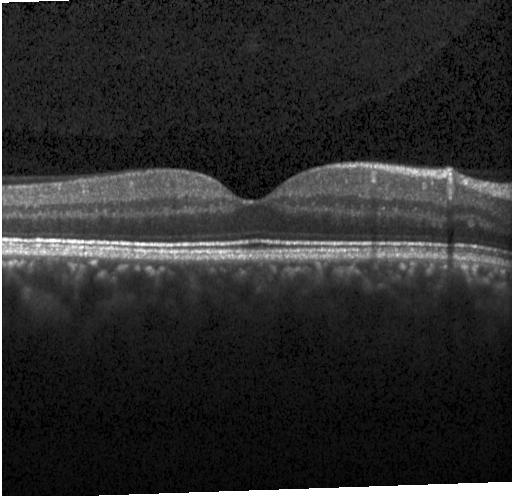
Spectral-domain optical coherence tomography; OCT line scan; horizontal scan through the fovea. Assessment: no choroidal neovascularization, no diabetic macular edema, and no drusen.